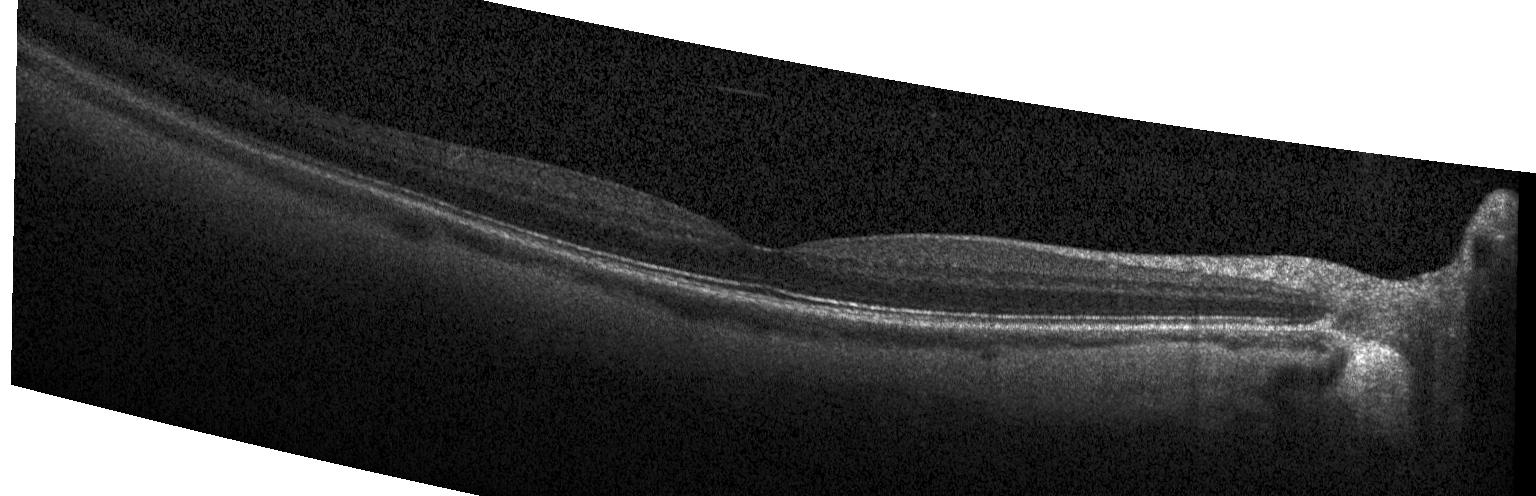 Neither CNV, DME, nor drusen.